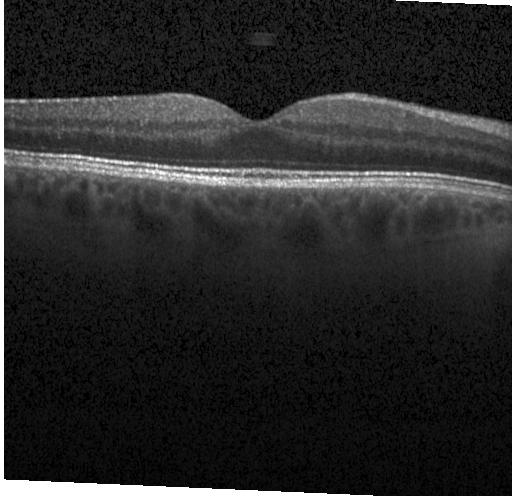
Retinal OCT cross-section, acquired on a Heidelberg Spectralis, fovea-centered, SD-OCT.
Finding: no choroidal neovascularization, no diabetic macular edema, and no drusen.